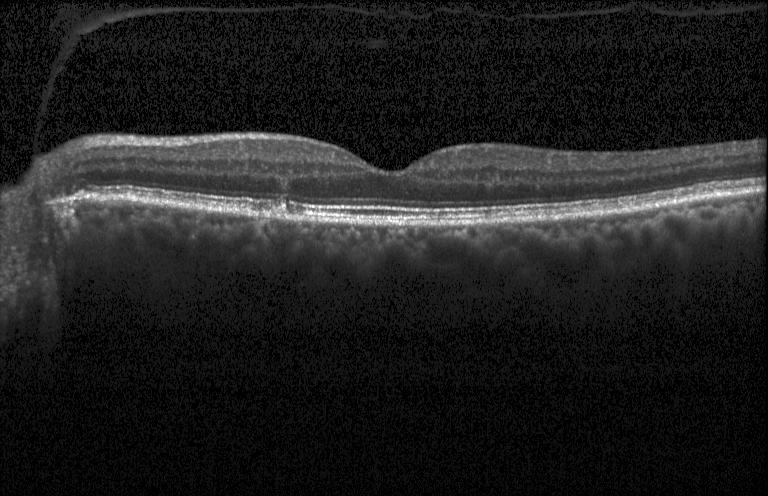
The scan shows drusen.